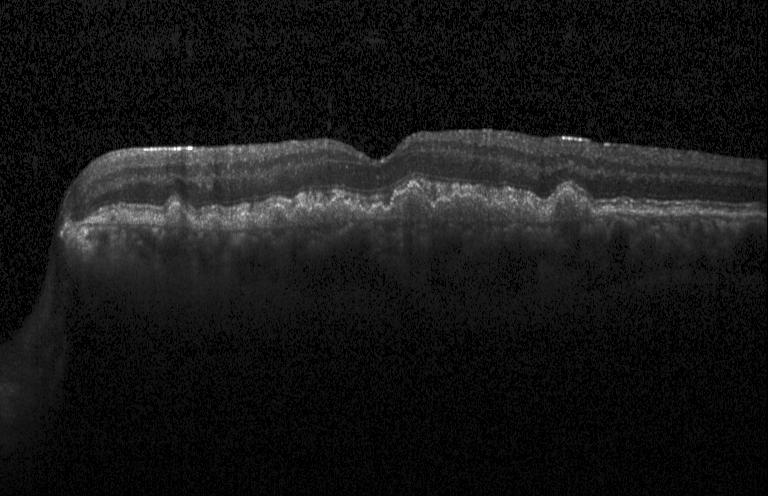

Retinal OCT cross-section · fovea-centered · Heidelberg Spectralis OCT system — Impression: a choroidal neovascular membrane.